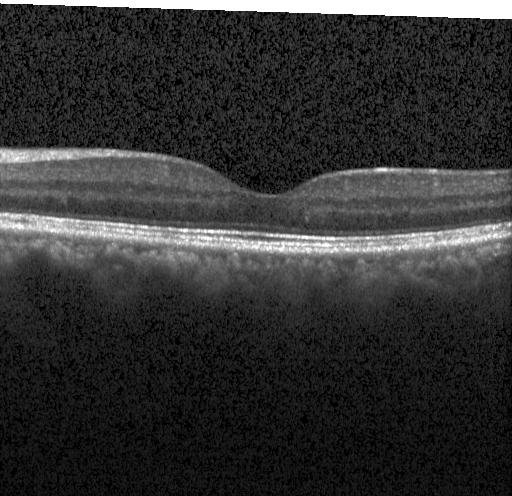

OCT finding: no choroidal neovascularization, diabetic macular edema, or drusen.